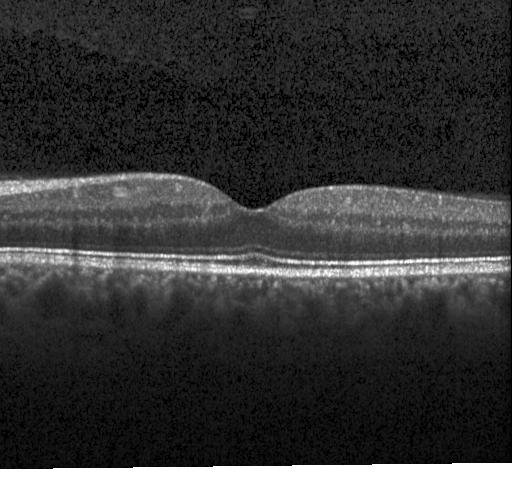
Macular scan, optical coherence tomography scan — Impression: neither CNV, DME, nor drusen.